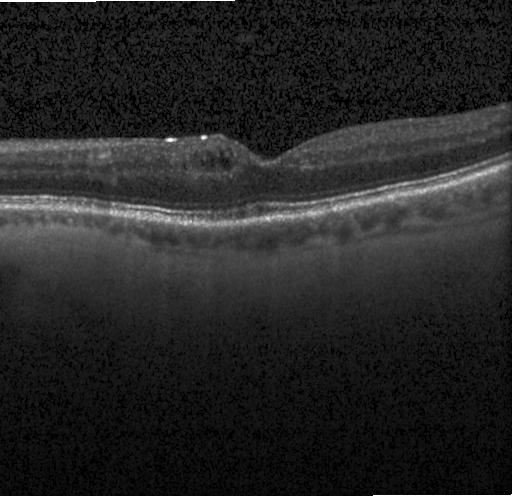

Finding: diabetic macular edema.